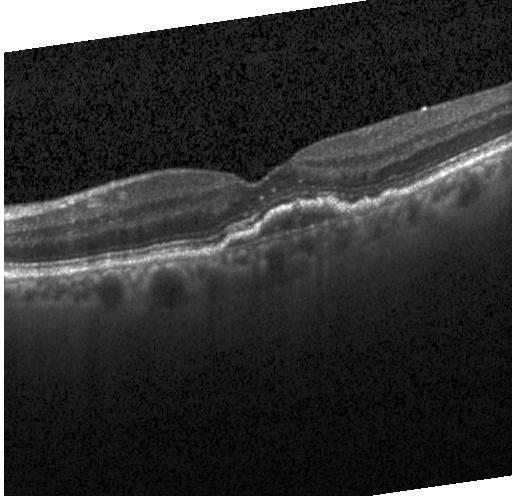
Diagnosis: choroidal neovascularization.